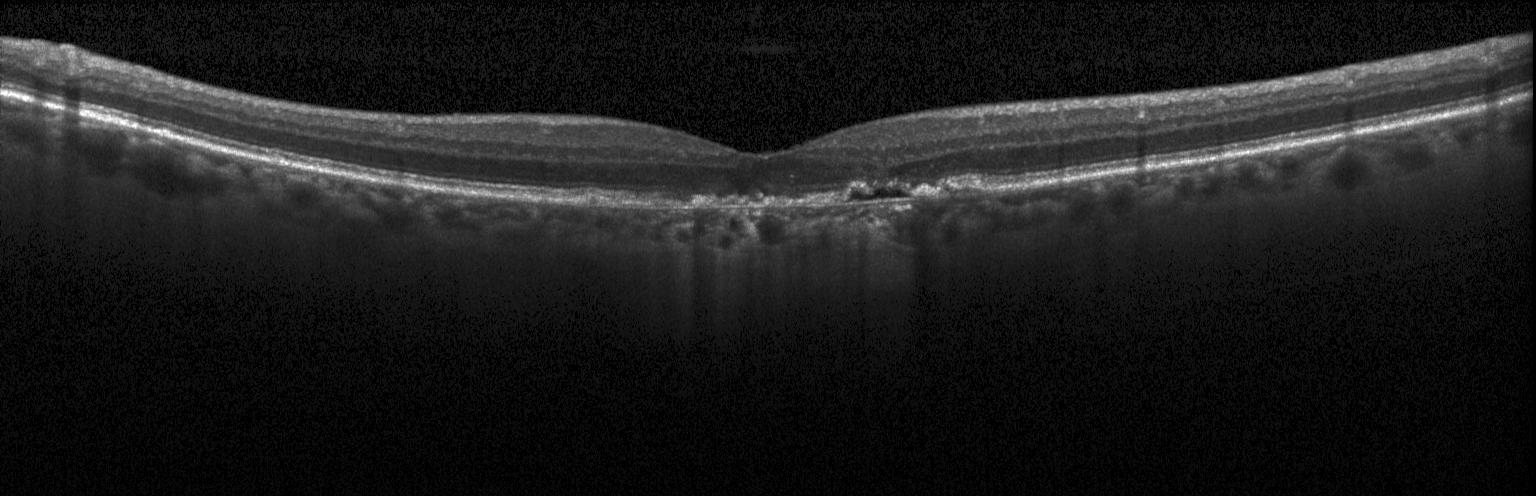
Spectral-domain OCT B-scan: a choroidal neovascular membrane.